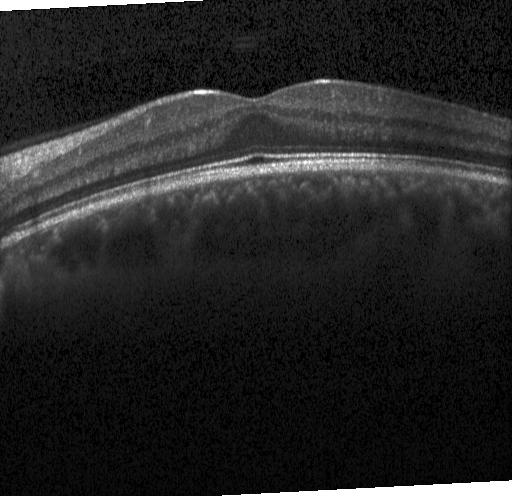
Acquired on a Heidelberg Spectralis, optical coherence tomography scan, spectral-domain OCT, through the macula — Diagnosis: no evidence of choroidal neovascularization, diabetic macular edema, or drusen.